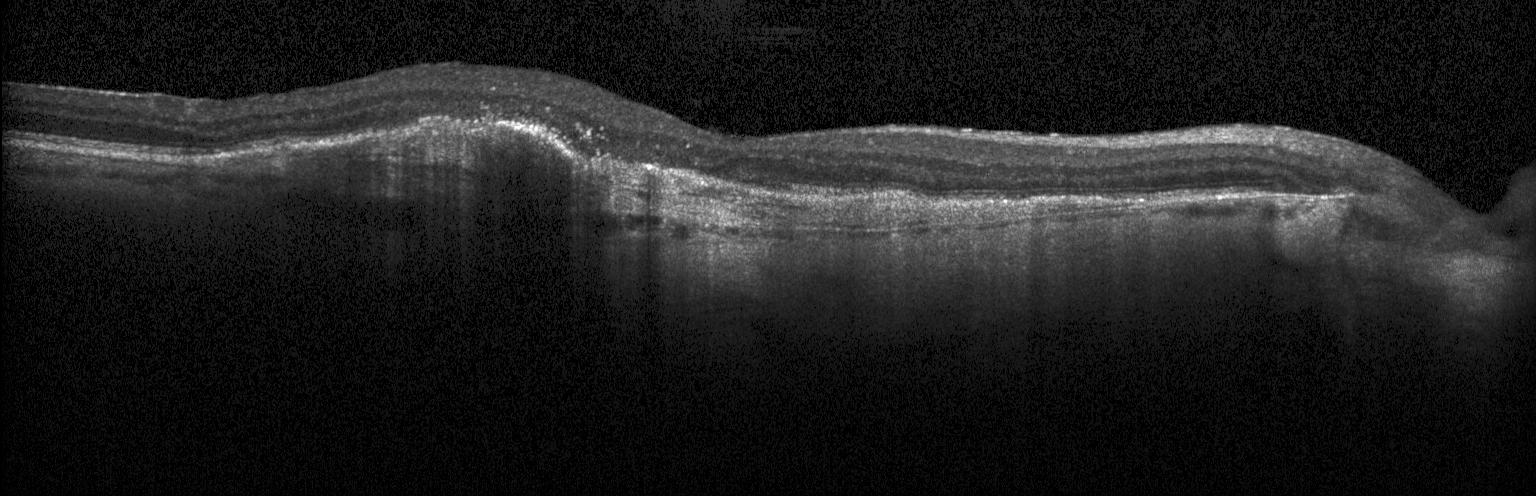 Finding: choroidal neovascularization.